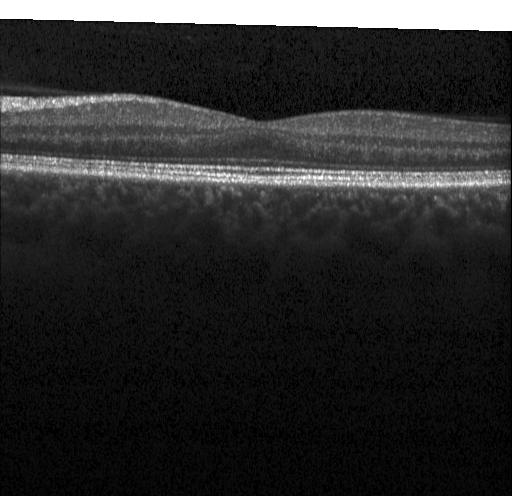
This B-scan demonstrates no choroidal neovascularization, diabetic macular edema, or drusen.